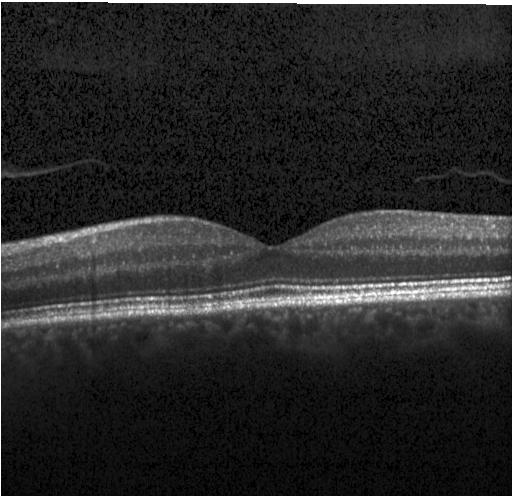

Heidelberg Spectralis, optical coherence tomography scan, centered on the fovea, spectral-domain optical coherence tomography
The scan shows no evidence of choroidal neovascularization, diabetic macular edema, or drusen.